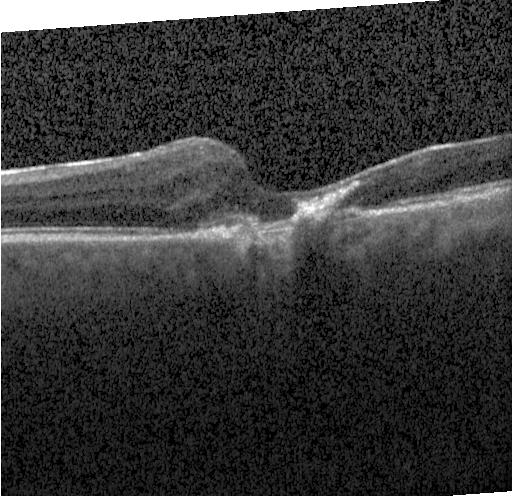

Fovea-centered. Retinal OCT cross-section — Diagnosis: choroidal neovascularization.